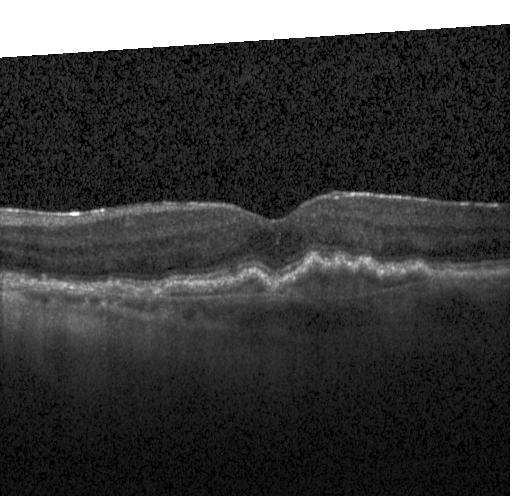

Spectral-domain optical coherence tomography, optical coherence tomography scan.
Assessment: a choroidal neovascular membrane.